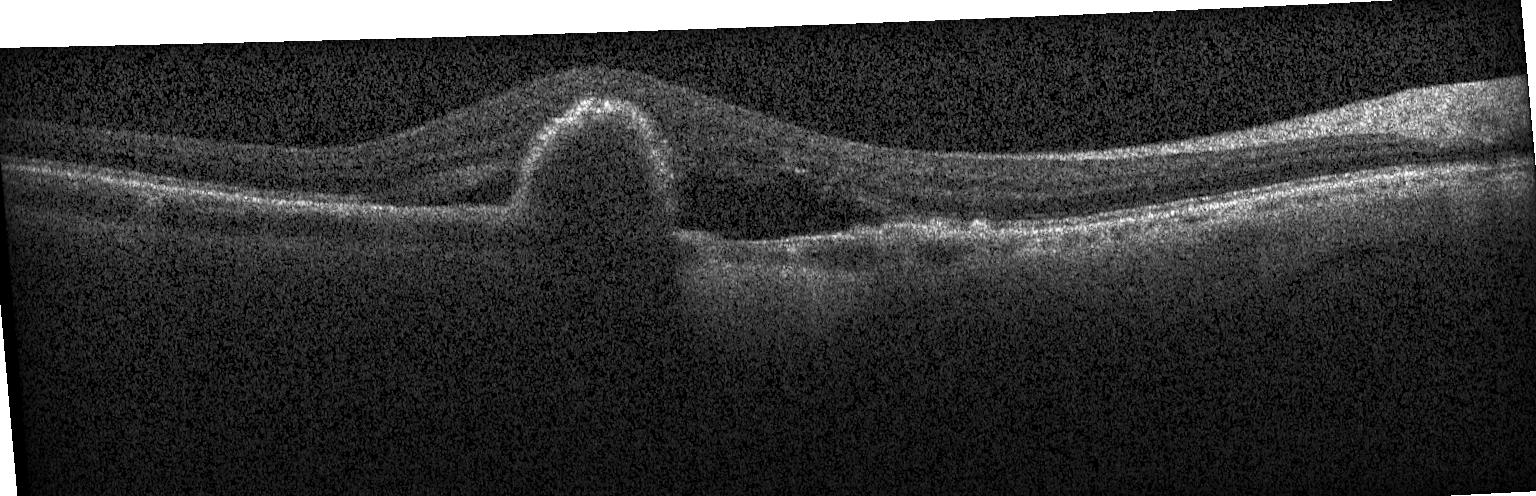

OCT B-scan showing choroidal neovascularization.